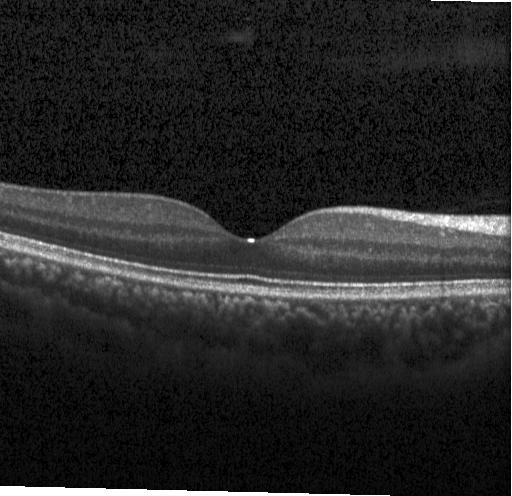
OCT finding: no choroidal neovascularization, no diabetic macular edema, and no drusen.